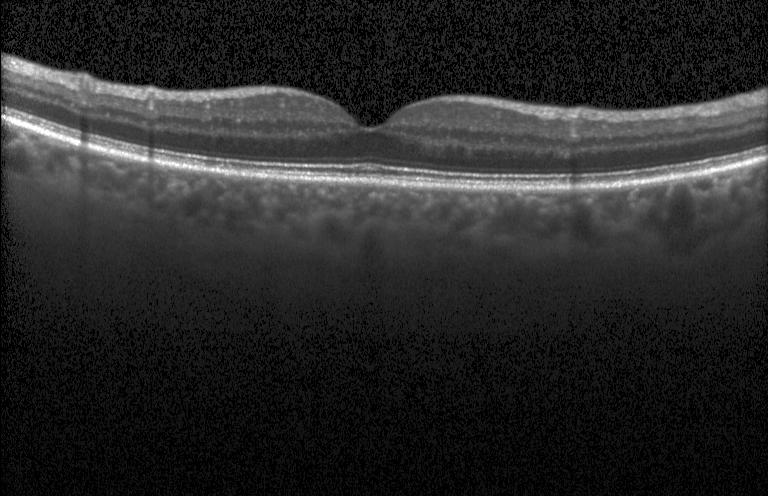 Impression: no evidence of choroidal neovascularization, diabetic macular edema, or drusen.